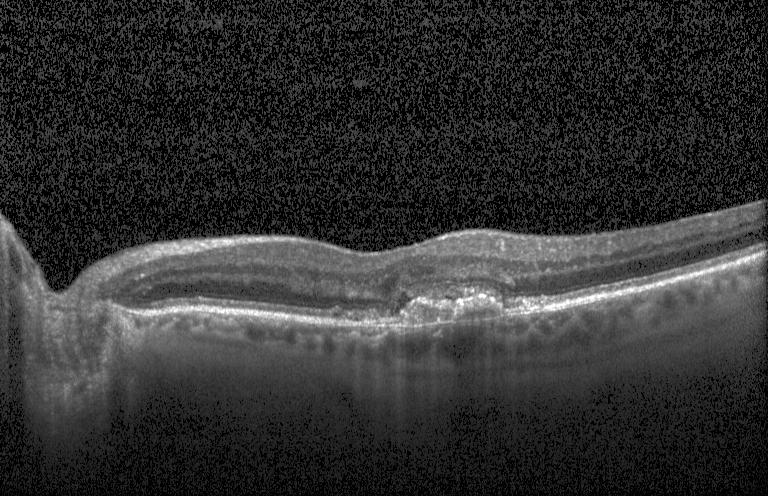

Finding: a choroidal neovascular membrane.